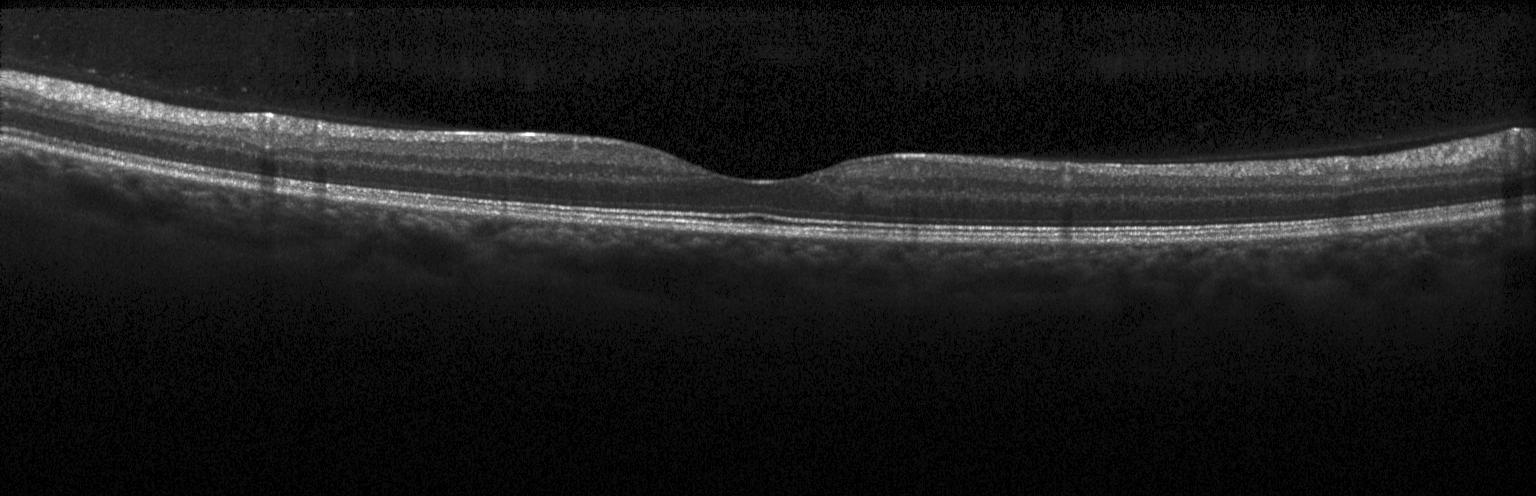 Optical coherence tomography scan.
No evidence of choroidal neovascularization, diabetic macular edema, or drusen.